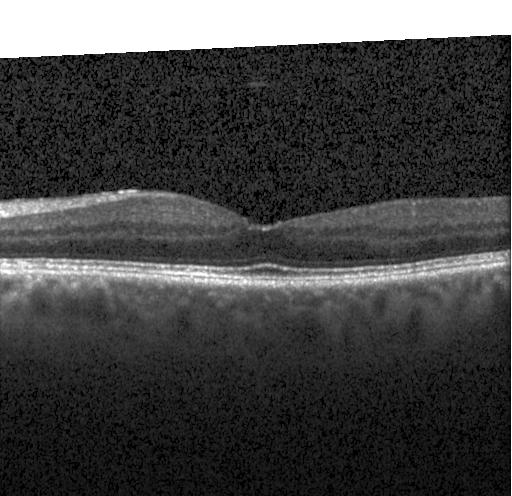 Heidelberg Spectralis. Optical coherence tomography B-scan
Macular OCT: no CNV, DME, or drusen.